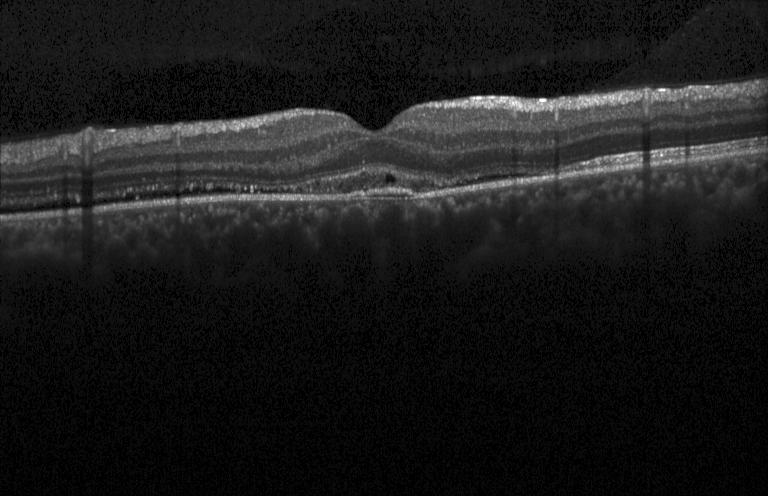
OCT line scan — The scan shows choroidal neovascularization.